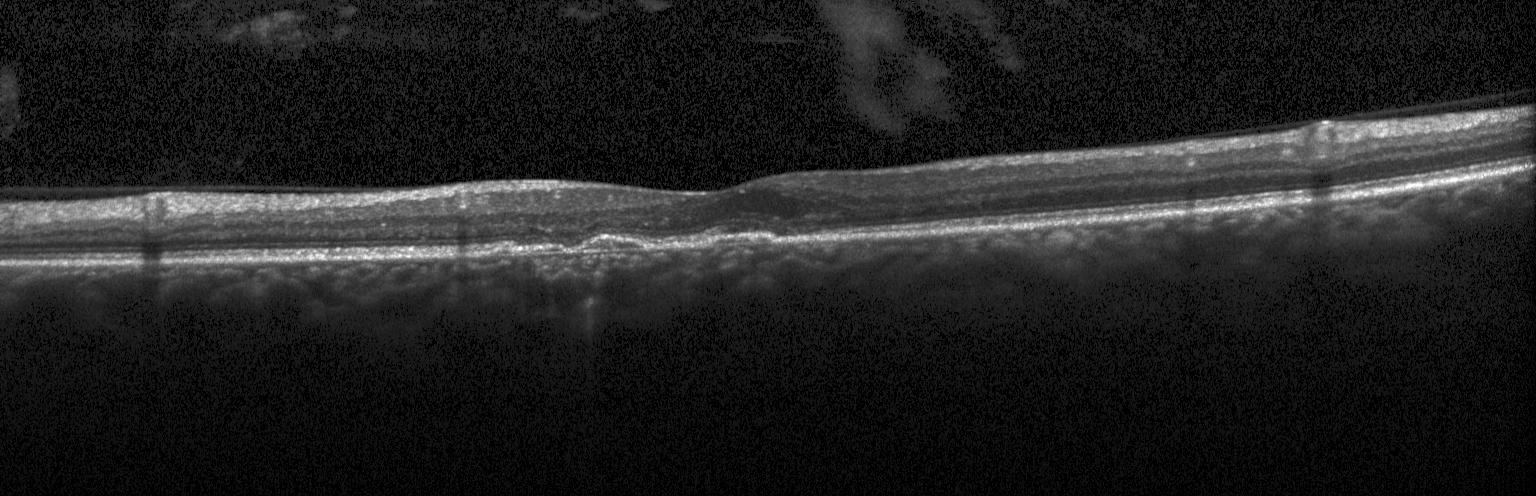

Spectral-domain OCT B-scan: a choroidal neovascular membrane.